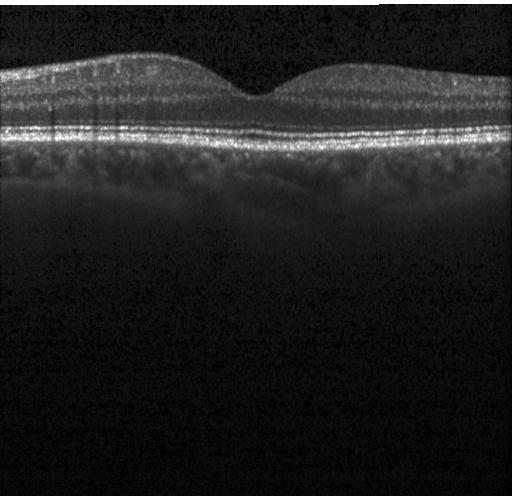

Finding: neither CNV, DME, nor drusen.